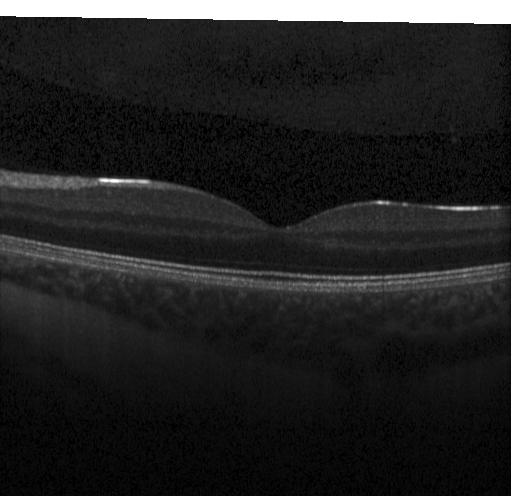

The scan shows no choroidal neovascularization, no diabetic macular edema, and no drusen.